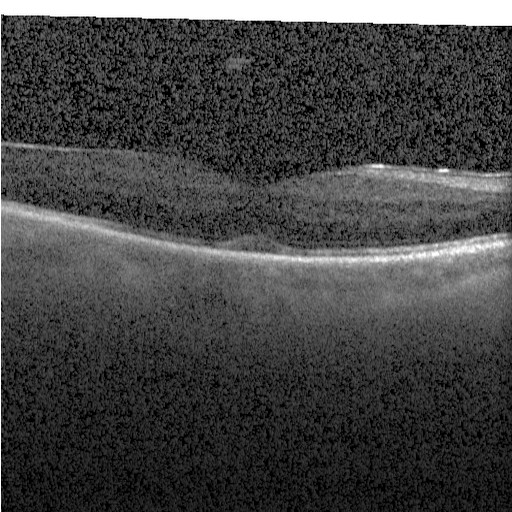

Macular OCT: DME.